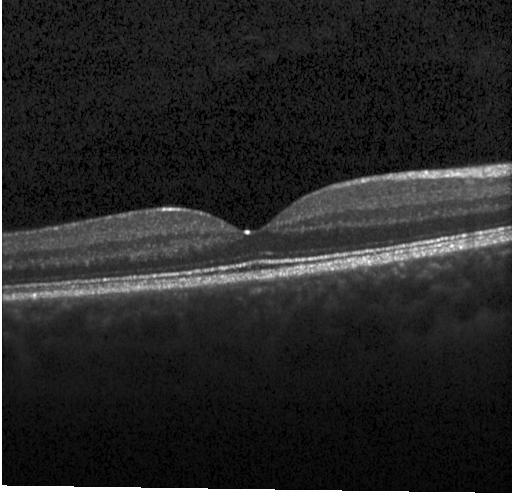
Diagnosis: neither choroidal neovascularization, diabetic macular edema, nor drusen.